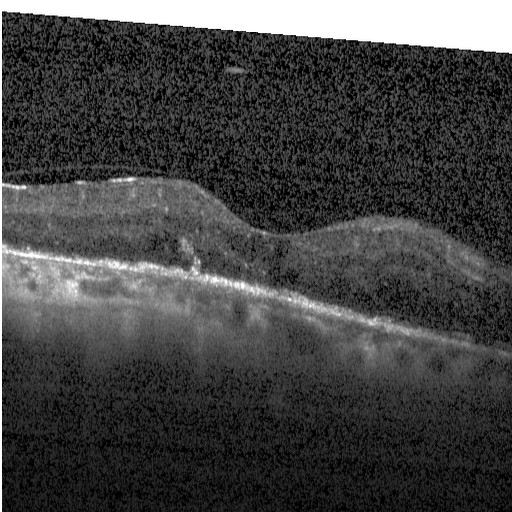

Optical coherence tomography B-scan
Finding: DME.